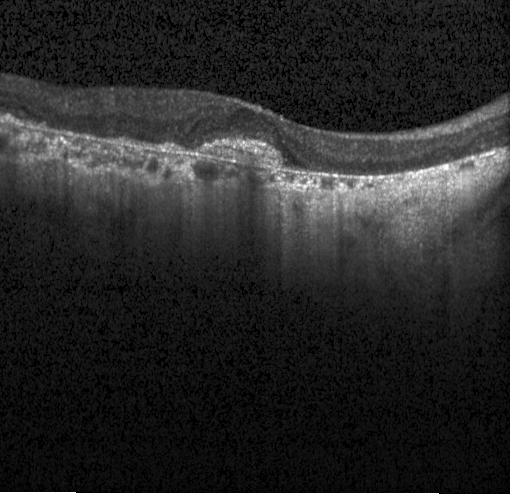

Optical coherence tomography B-scan; SD-OCT; through the macula
Finding: a choroidal neovascular membrane.